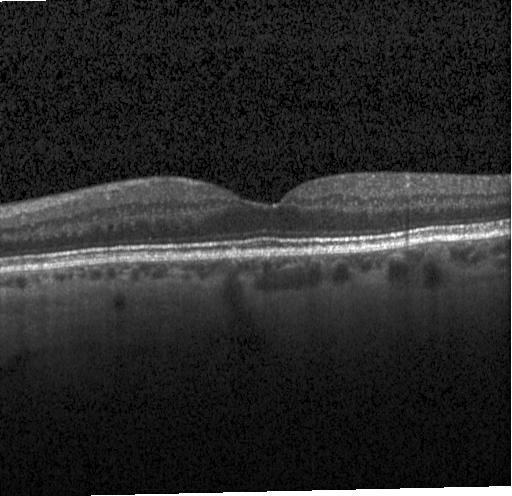

Spectral-domain OCT · instrument: Heidelberg Spectralis · optical coherence tomography B-scan · fovea-centered — Macular OCT: neither choroidal neovascularization, diabetic macular edema, nor drusen.